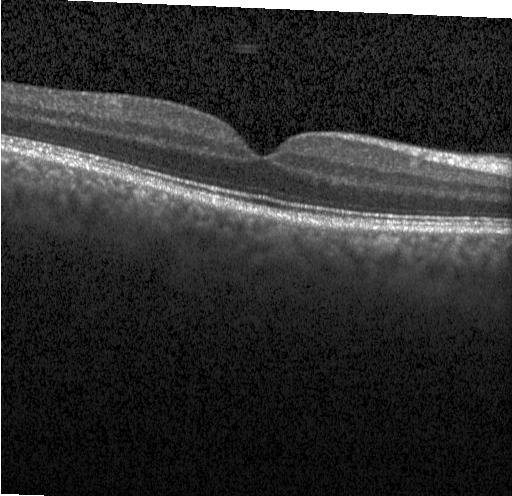
Diagnosis: no choroidal neovascularization, no diabetic macular edema, and no drusen.